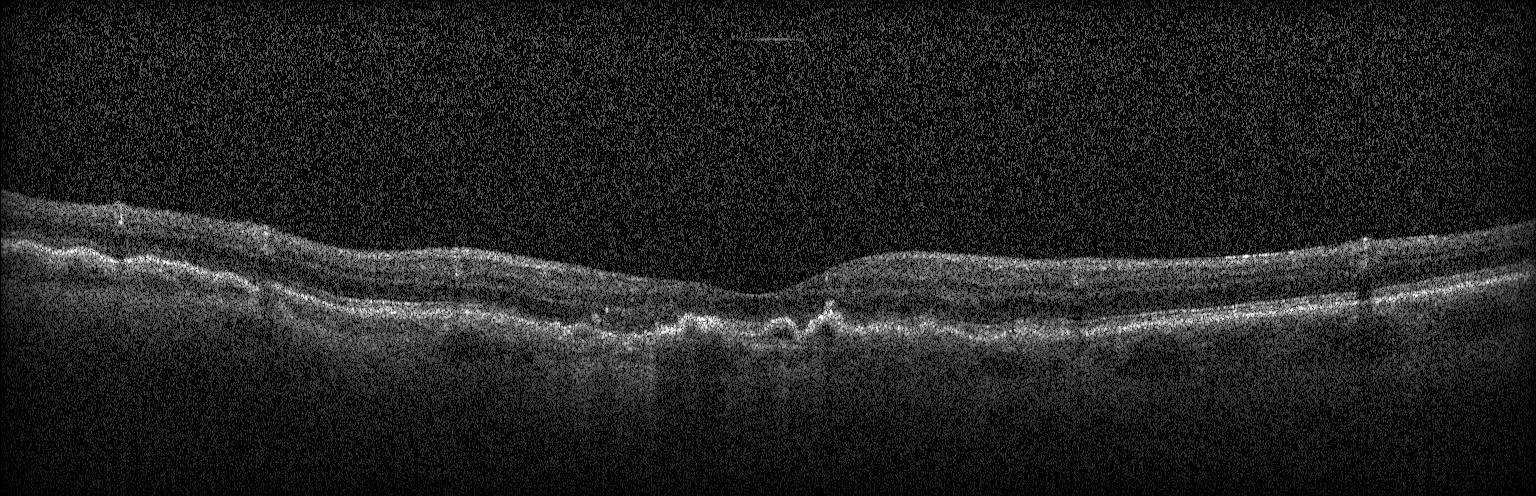

Finding: choroidal neovascularization (CNV).